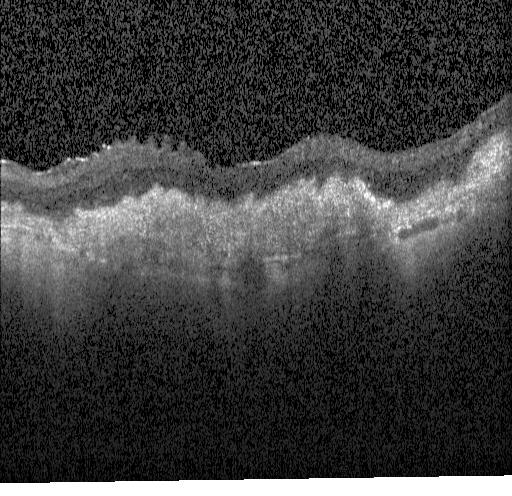 Macular OCT: choroidal neovascularization.